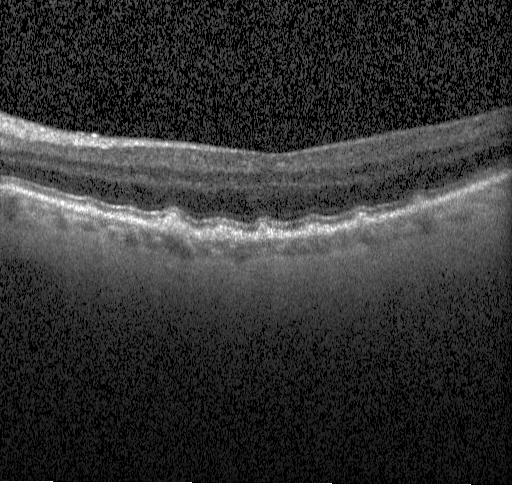
Optical coherence tomography scan · fovea-centered.
Impression: drusen.